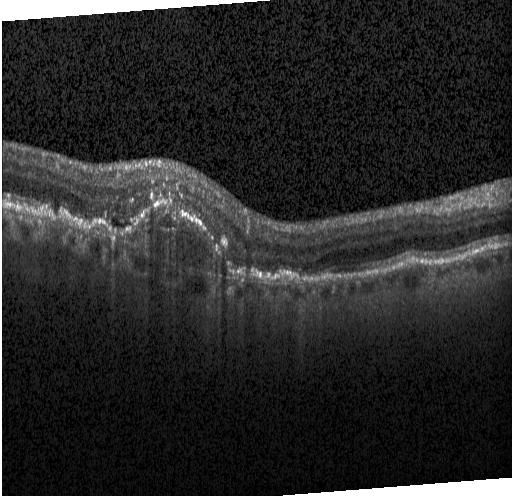

Retinal OCT B-scan; Heidelberg Spectralis OCT system.
Dx: CNV.